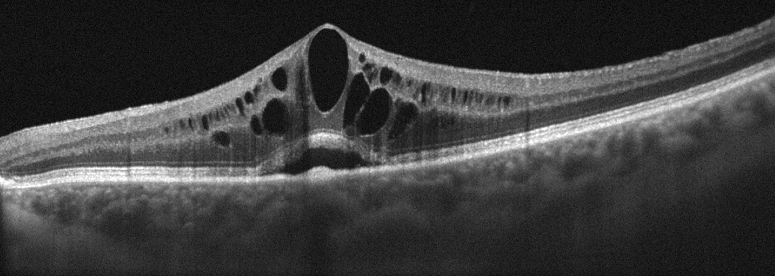 Oculus sinister; OCT line scan. Finding: retinal vein occlusion.